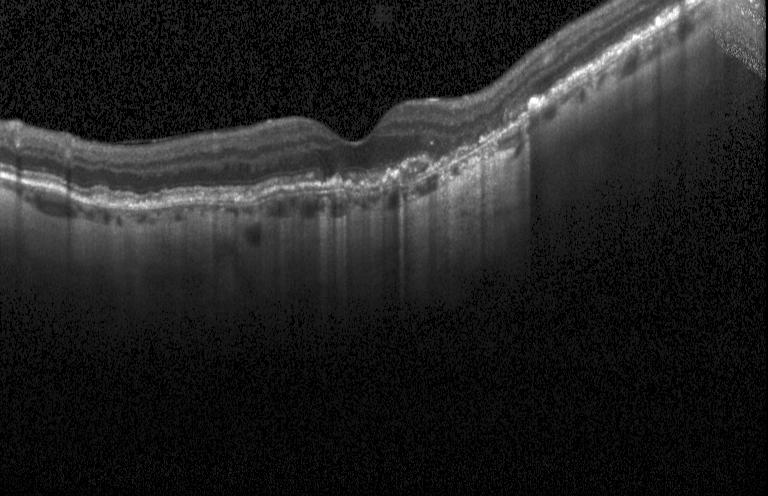 Retinal OCT B-scan.
Dx: choroidal neovascularization.